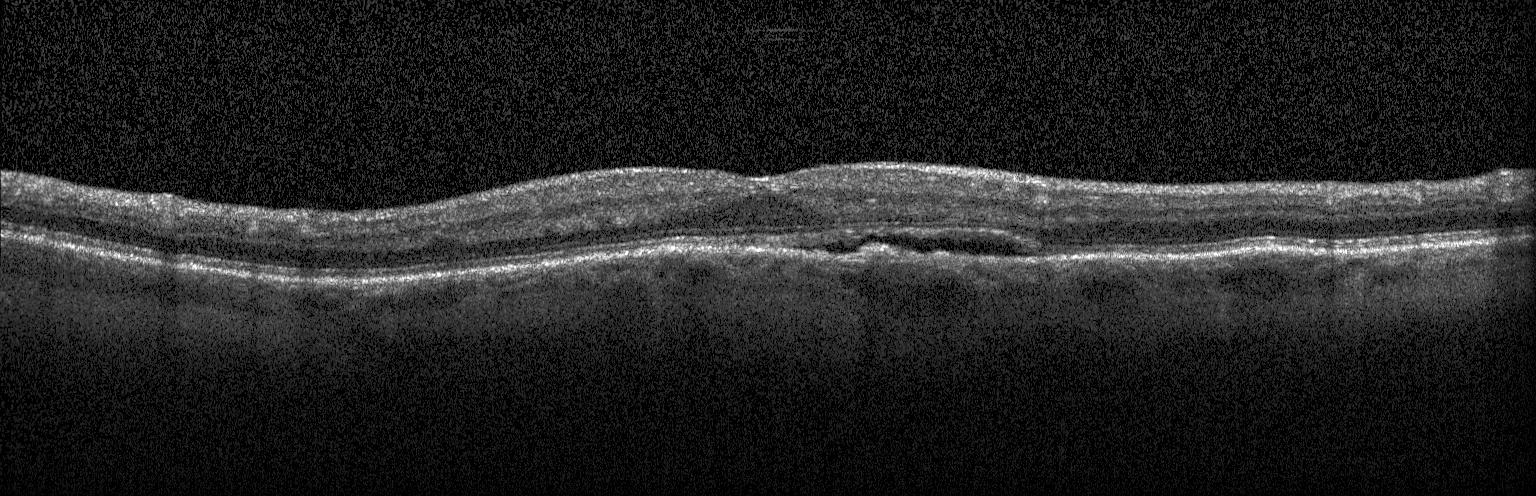 OCT line scan
Diagnosis: a choroidal neovascular membrane.